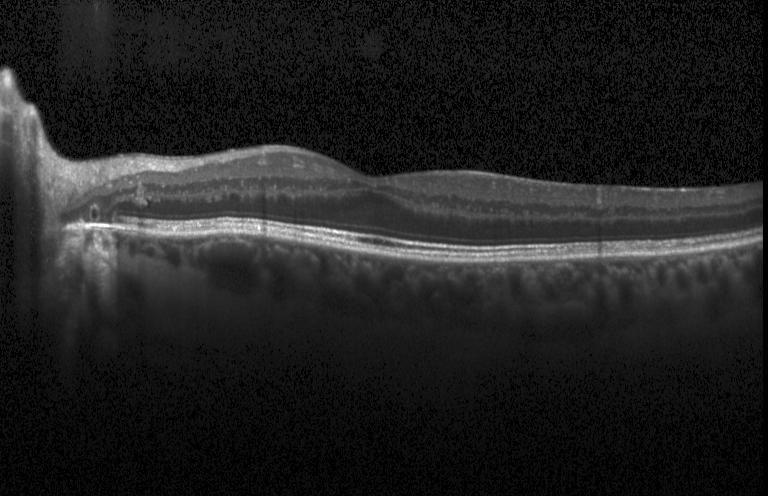
Retinal OCT cross-section showing no choroidal neovascularization, diabetic macular edema, or drusen.